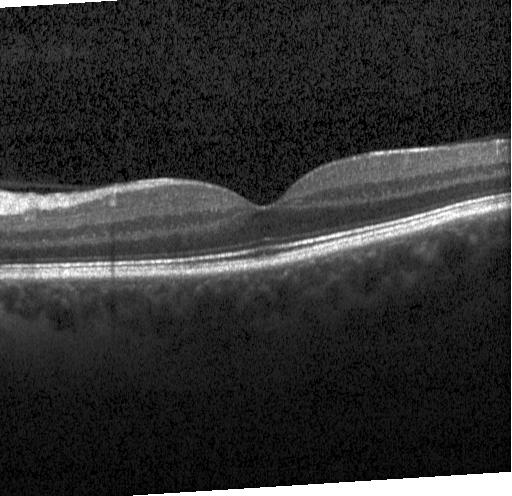 Spectral-domain optical coherence tomography · retinal OCT cross-section · instrument: Heidelberg Spectralis · centered on the fovea.
Dx: no evidence of choroidal neovascularization, diabetic macular edema, or drusen.